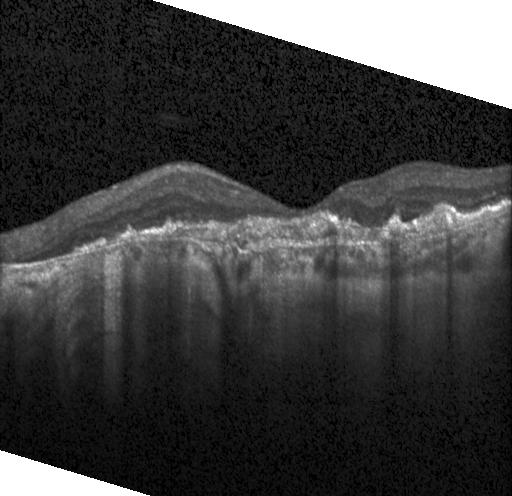

OCT line scan. CNV.